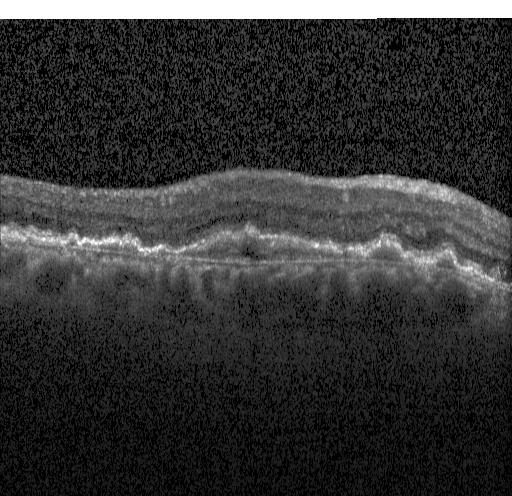 SD-OCT · OCT B-scan · fovea-centered
Macular OCT: choroidal neovascularization (CNV).